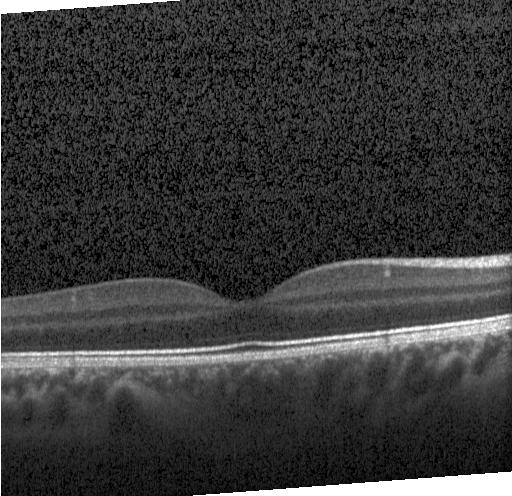
Macular OCT demonstrating no choroidal neovascularization, no diabetic macular edema, and no drusen.